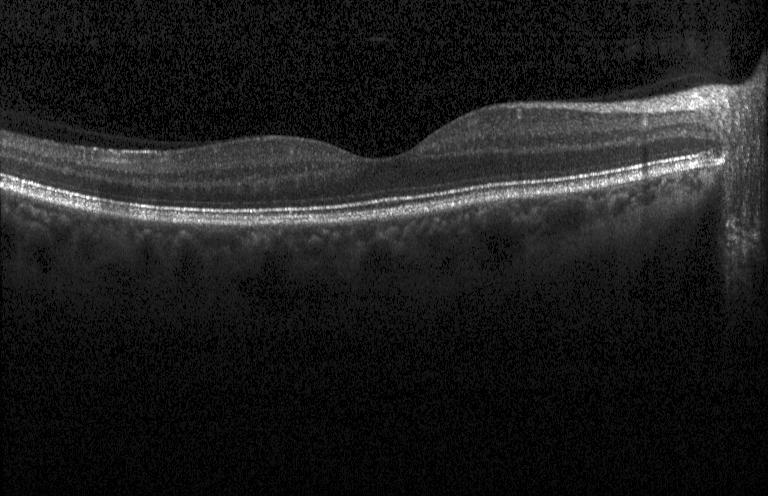 Horizontal scan through the fovea; retinal OCT cross-section
OCT finding: neither CNV, DME, nor drusen.